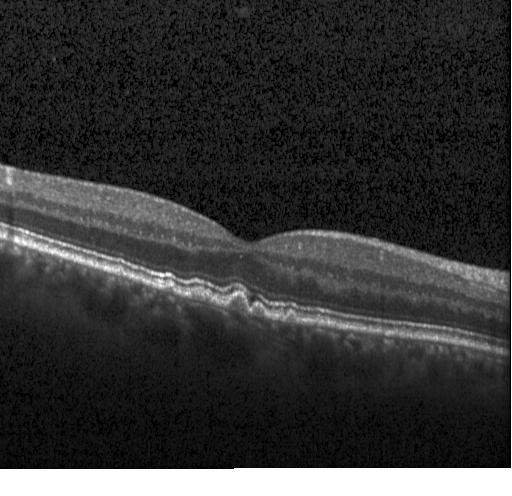 Optical coherence tomography scan — Impression: drusen.